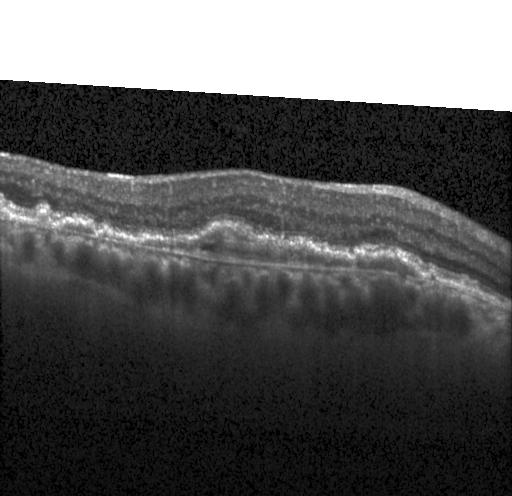

Spectral-domain optical coherence tomography · OCT line scan · macular scan · Heidelberg Spectralis.
Macular OCT: CNV.